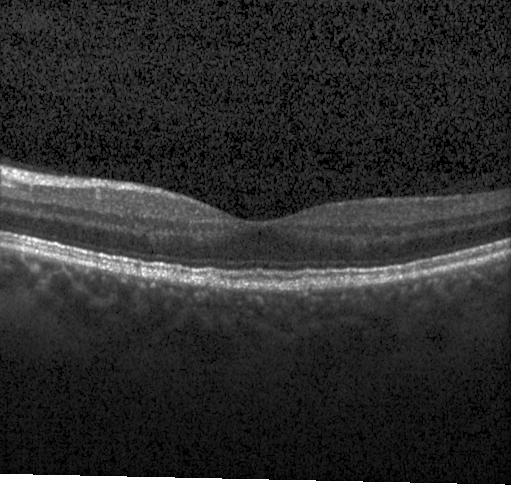

Finding: neither choroidal neovascularization, diabetic macular edema, nor drusen.